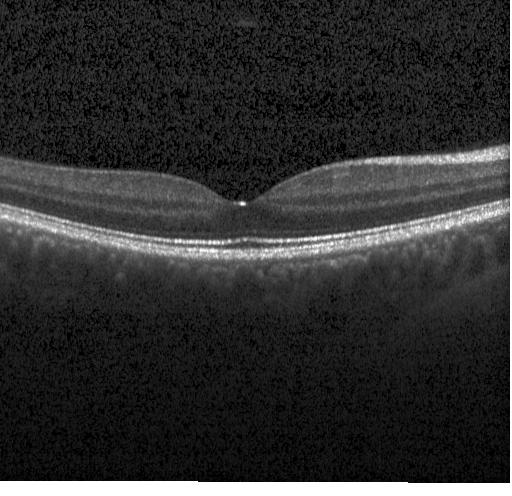 OCT line scan. Heidelberg Spectralis. Macular scan. Spectral-domain optical coherence tomography. Diagnosis: no CNV, DME, or drusen.